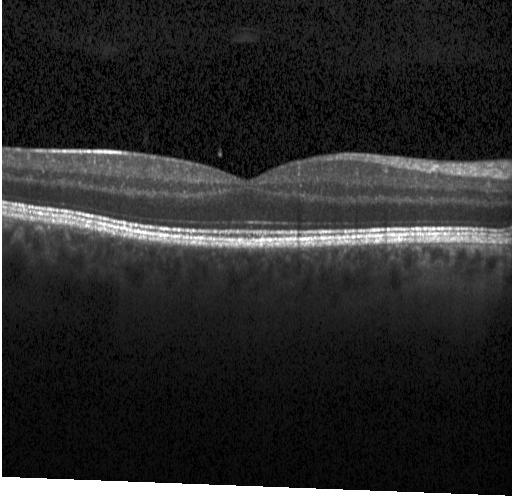

Dx: no CNV, DME, or drusen.